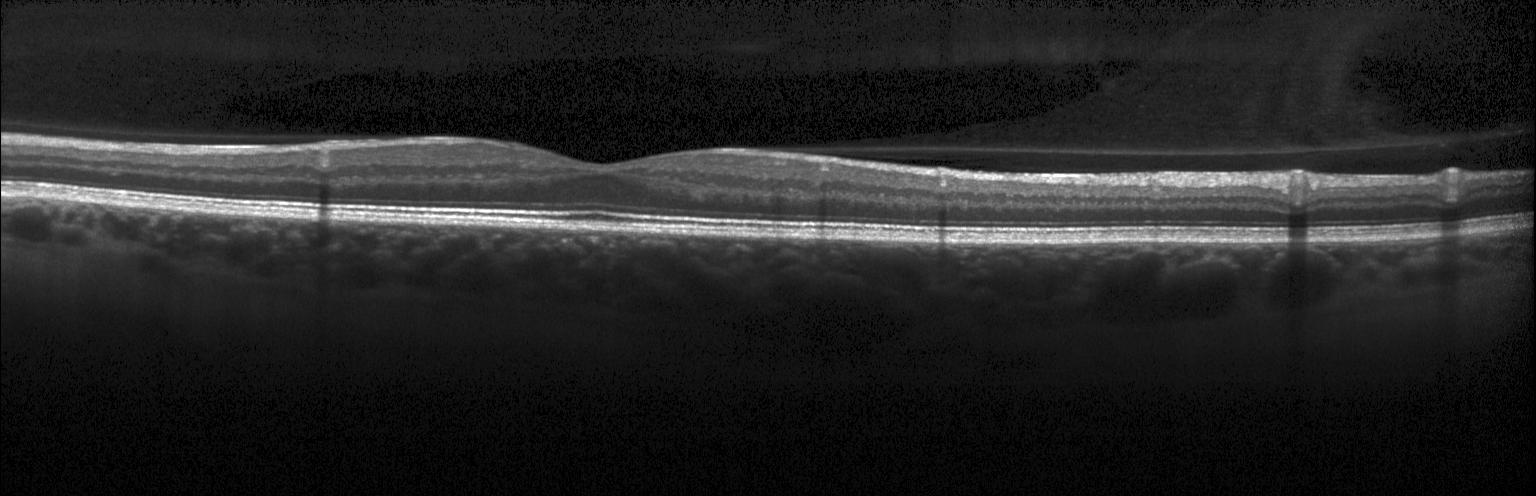

Retinal OCT B-scan.
Neither CNV, DME, nor drusen.